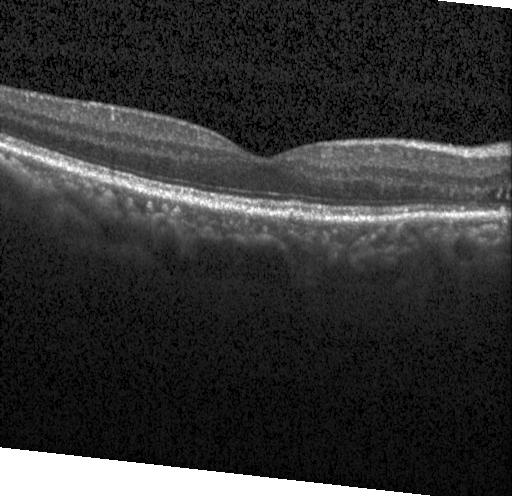
OCT scan showing neither choroidal neovascularization, diabetic macular edema, nor drusen.